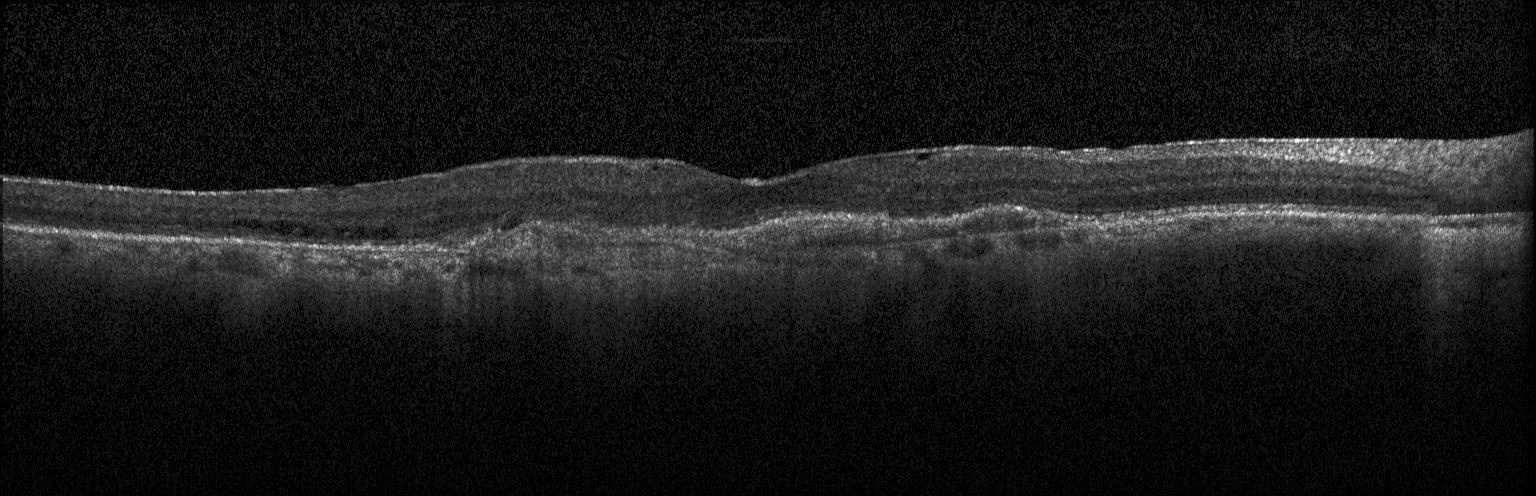 OCT B-scan
OCT finding: a choroidal neovascular membrane.